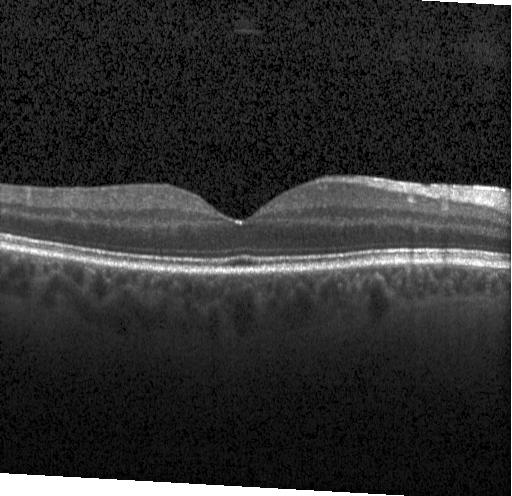 Spectral-domain OCT, instrument: Heidelberg Spectralis, horizontal scan through the fovea, optical coherence tomography scan.
Dx: neither choroidal neovascularization, diabetic macular edema, nor drusen.